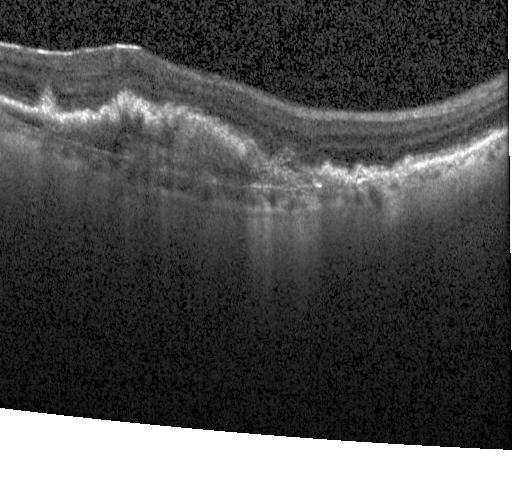
OCT line scan · horizontal scan through the fovea. Finding: CNV.